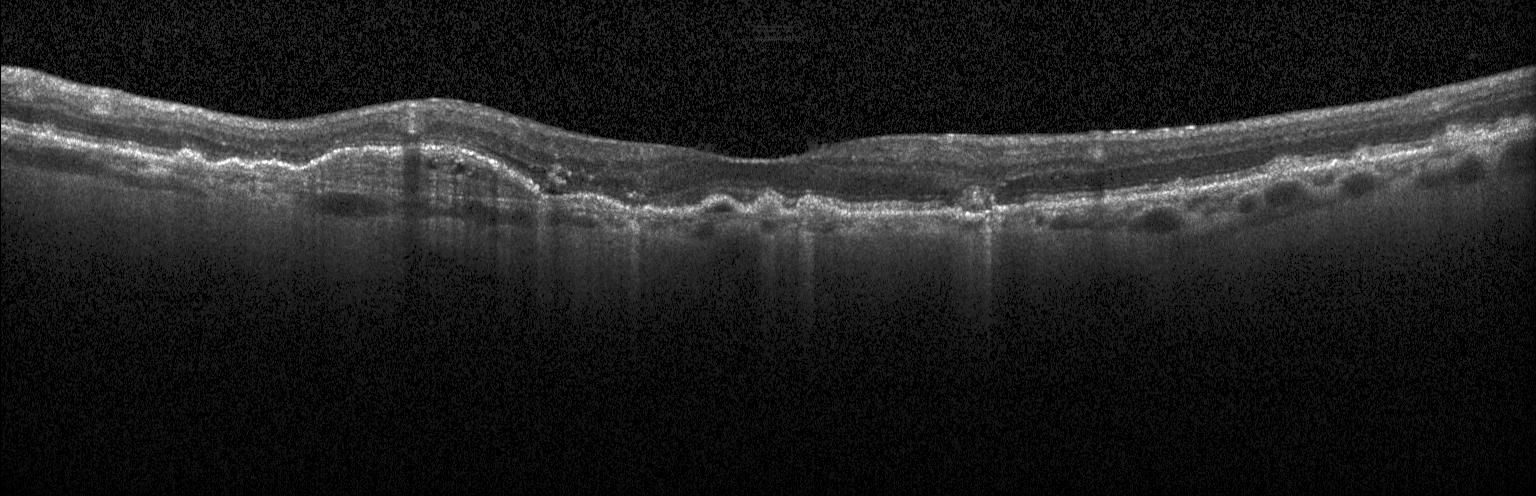

Retinal OCT cross-section. Macular OCT: choroidal neovascularization (CNV).